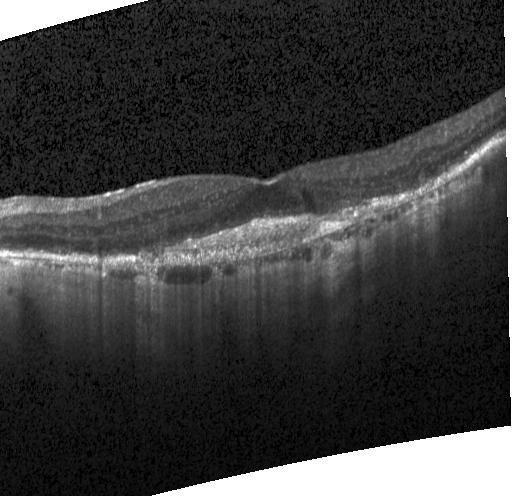

Through the macula; retinal OCT cross-section.
Finding: CNV.